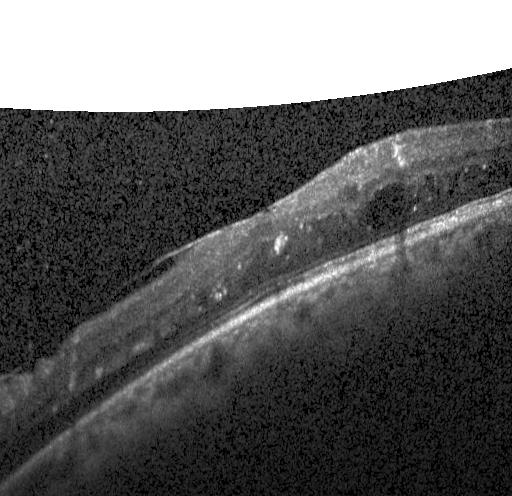
SD-OCT; OCT B-scan. Dx: diabetic macular edema (DME).